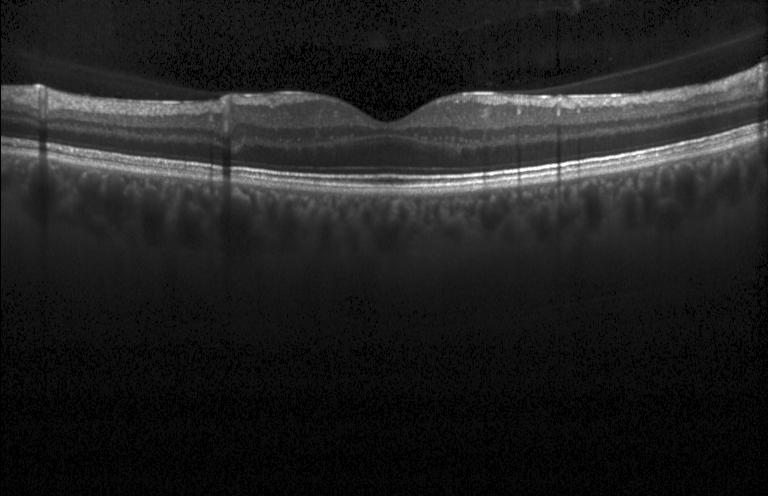

Impression: neither CNV, DME, nor drusen.